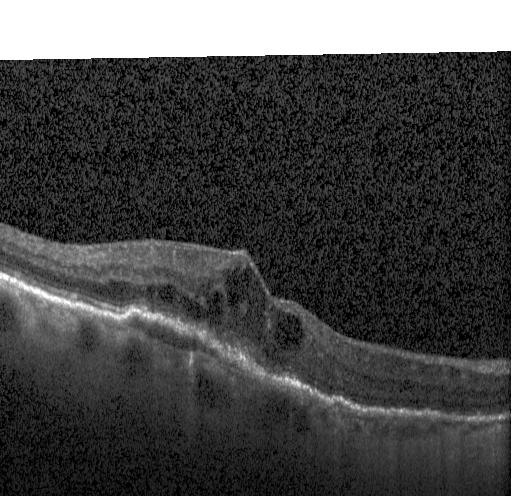
Through the macula. Spectral-domain optical coherence tomography. Optical coherence tomography B-scan. Acquired on a Heidelberg Spectralis — Dx: choroidal neovascularization (CNV).